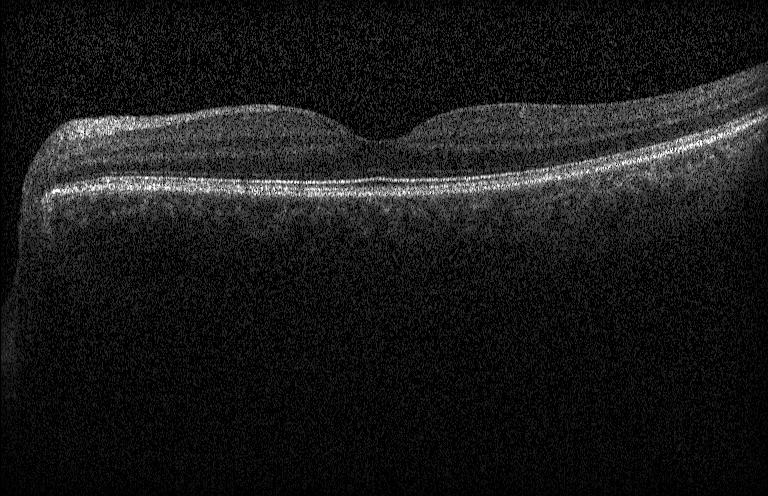
Horizontal scan through the fovea · optical coherence tomography B-scan · instrument: Heidelberg Spectralis. Diagnosis: no evidence of choroidal neovascularization, diabetic macular edema, or drusen.